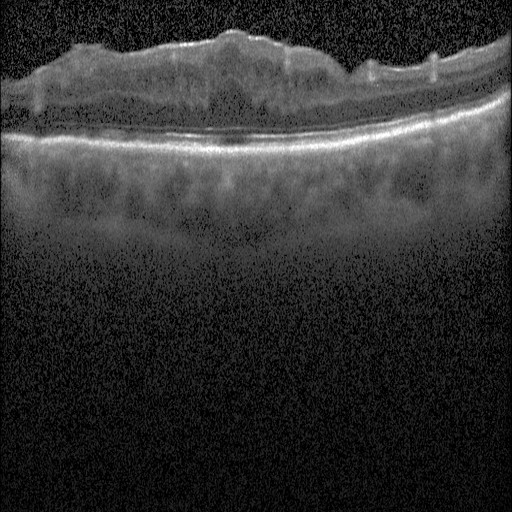
Instrument: Heidelberg Spectralis · spectral-domain OCT · macular scan · OCT B-scan
This B-scan demonstrates diabetic macular edema.